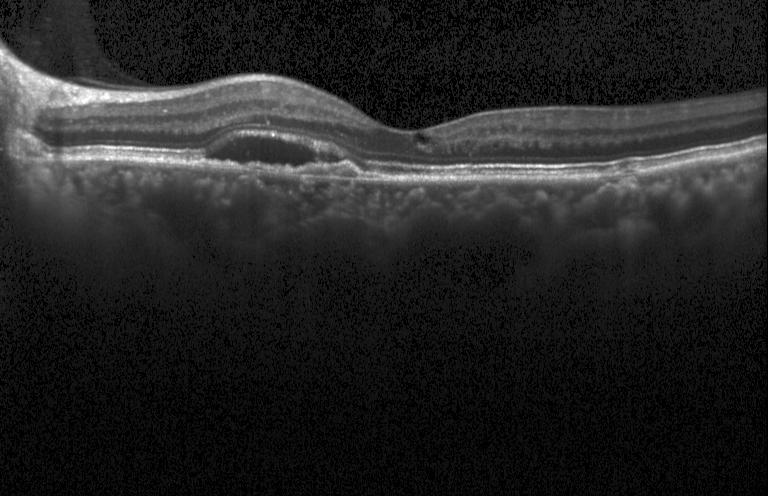
OCT B-scan, through the macula, SD-OCT. Dx: a choroidal neovascular membrane.